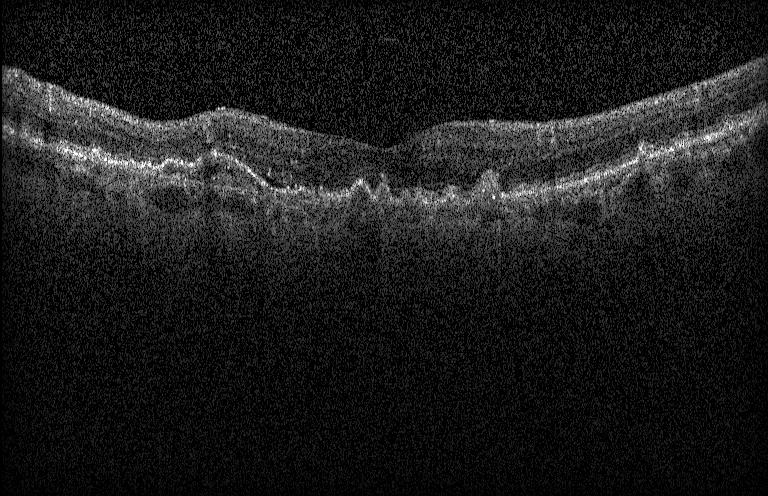
Assessment: a choroidal neovascular membrane.